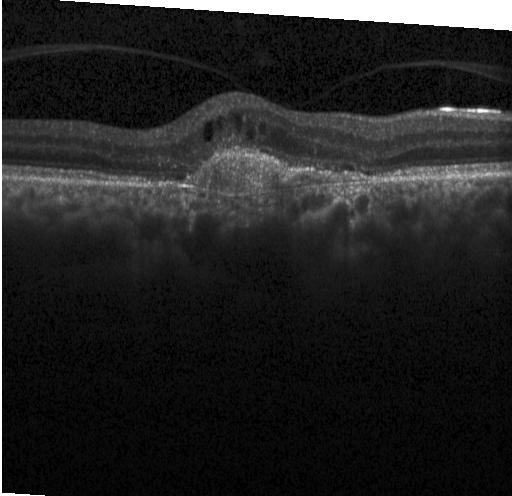
Retinal OCT cross-section.
Dx: a choroidal neovascular membrane.